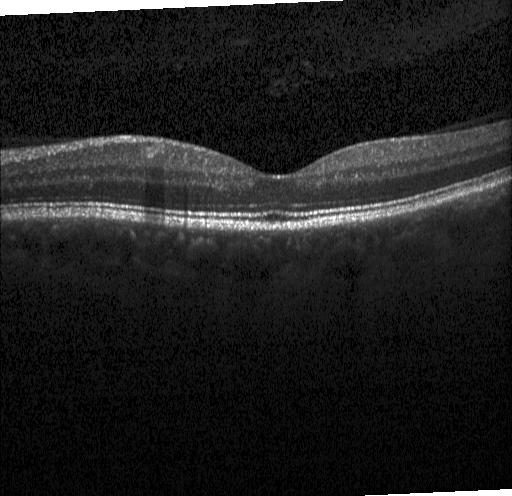

Spectral-domain optical coherence tomography, OCT B-scan, through the macula, Heidelberg Spectralis OCT system — Impression: no evidence of CNV, DME, or drusen.